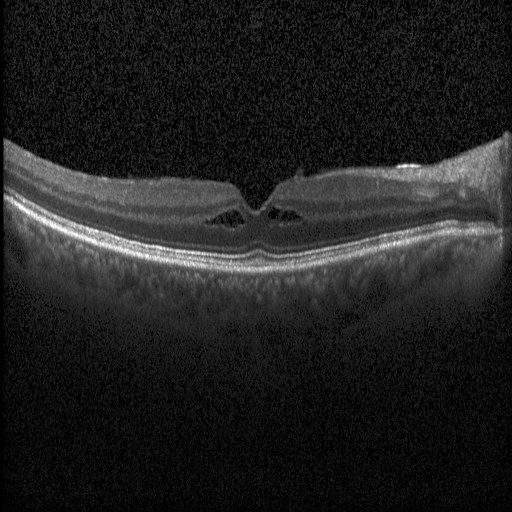 OCT line scan; instrument: Heidelberg Spectralis; SD-OCT; horizontal scan through the fovea — DME.